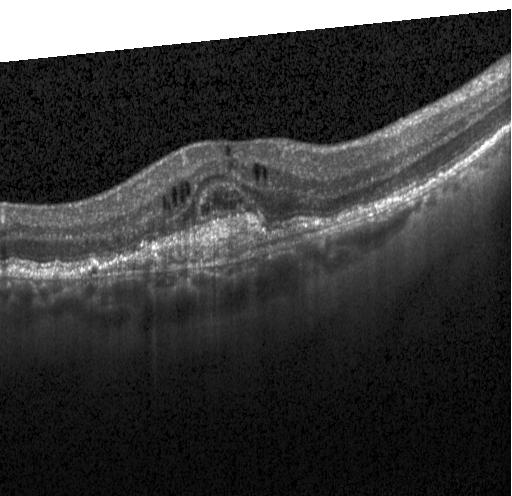 Spectral-domain OCT B-scan: a choroidal neovascular membrane.